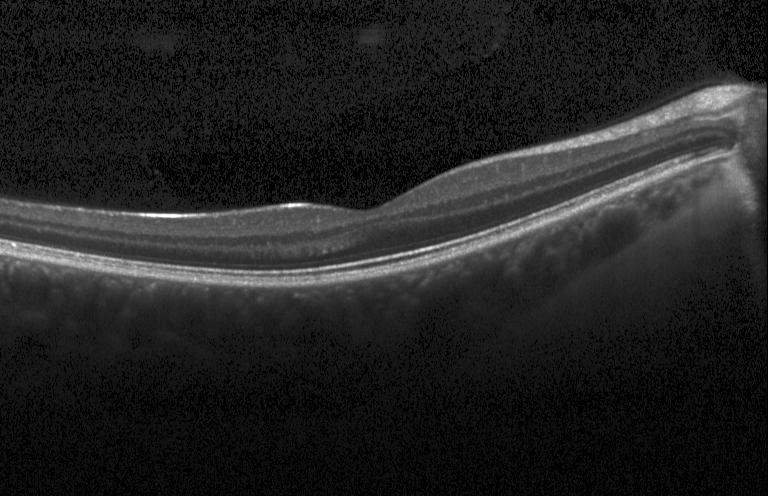

OCT B-scan. Heidelberg Spectralis. Finding: no choroidal neovascularization, diabetic macular edema, or drusen.